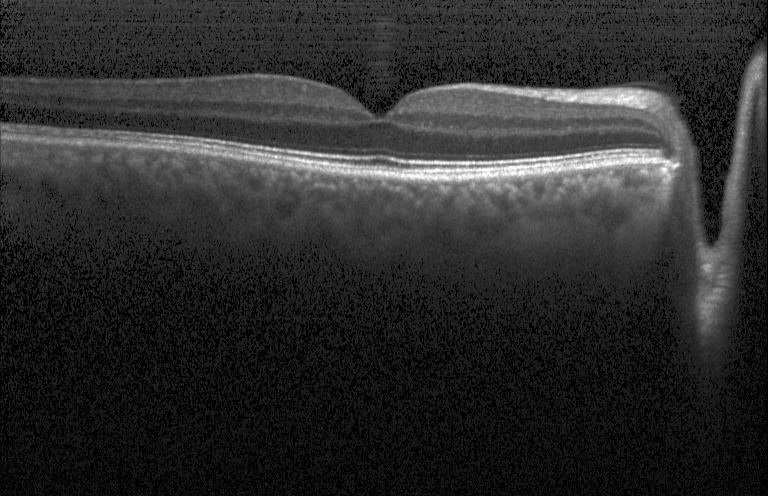

Horizontal scan through the fovea · acquired on a Heidelberg Spectralis · retinal OCT B-scan — OCT finding: neither CNV, DME, nor drusen.